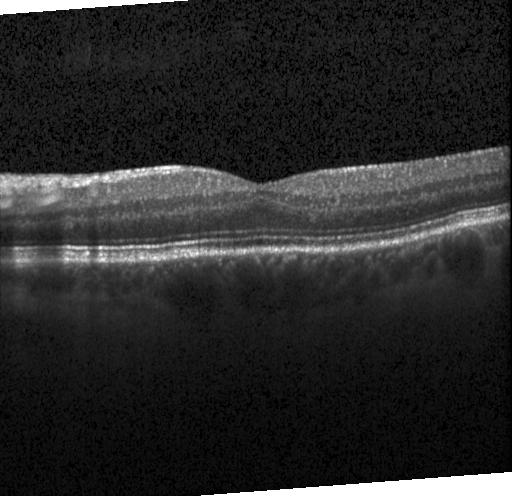

Spectral-domain OCT. Acquired on a Heidelberg Spectralis. Macular scan. Retinal OCT B-scan — Finding: neither choroidal neovascularization, diabetic macular edema, nor drusen.